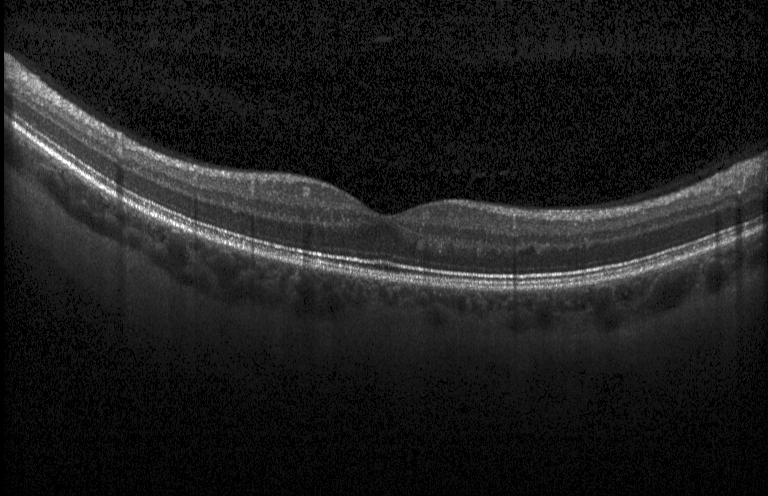

Retinal OCT B-scan · spectral-domain OCT
The scan shows no choroidal neovascularization, diabetic macular edema, or drusen.